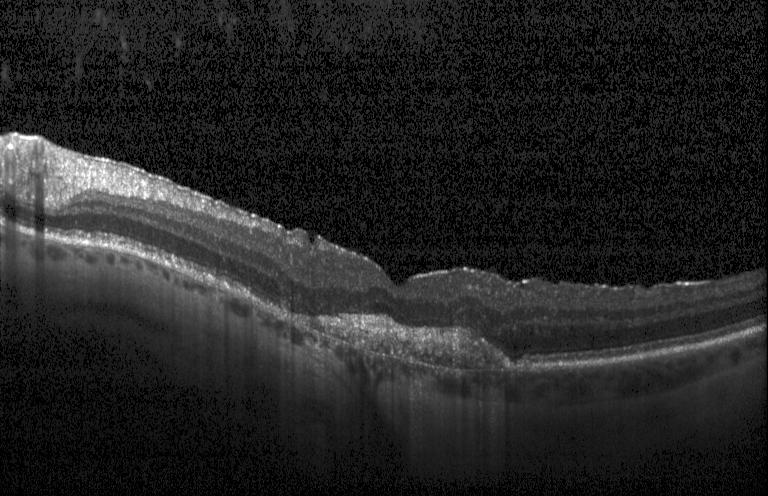

Fovea-centered. SD-OCT. Retinal OCT cross-section. Instrument: Heidelberg Spectralis. Finding: choroidal neovascularization (CNV).